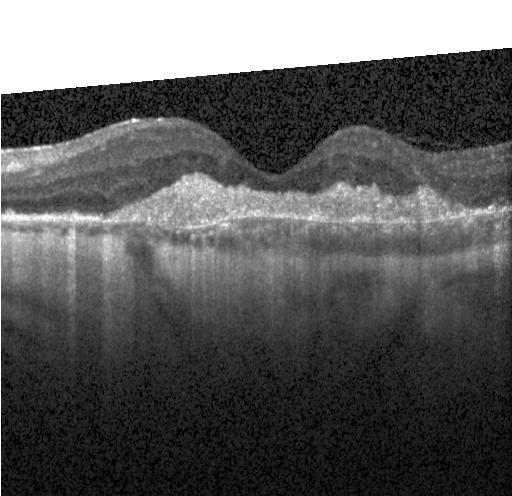
OCT finding: CNV.